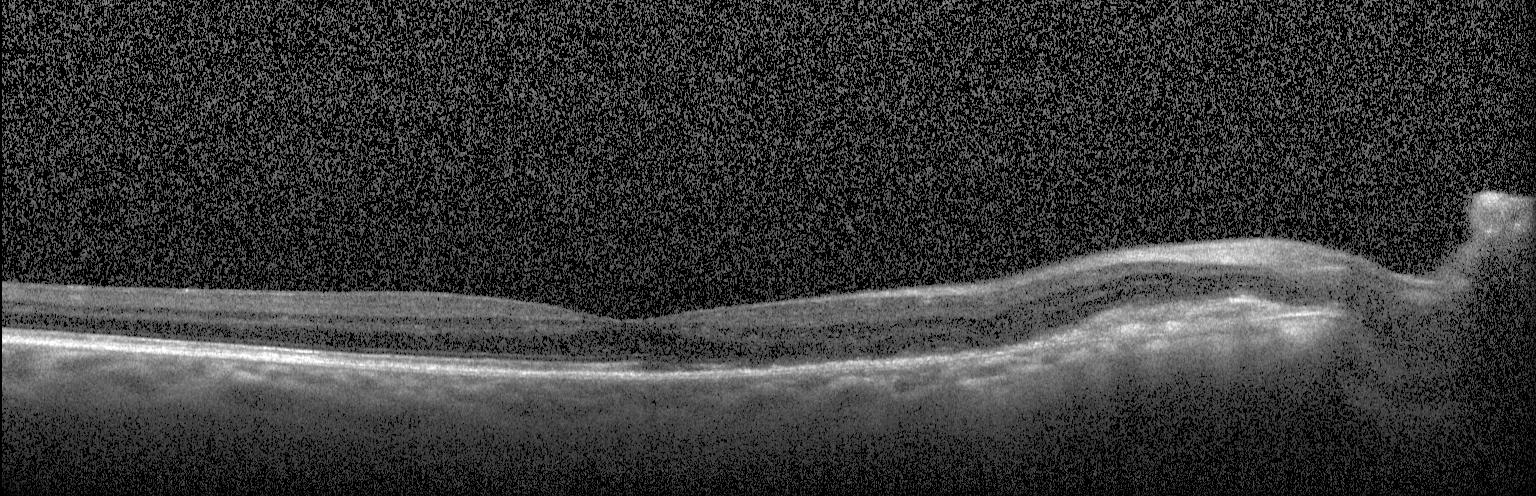

Optical coherence tomography scan
Diagnosis: CNV.